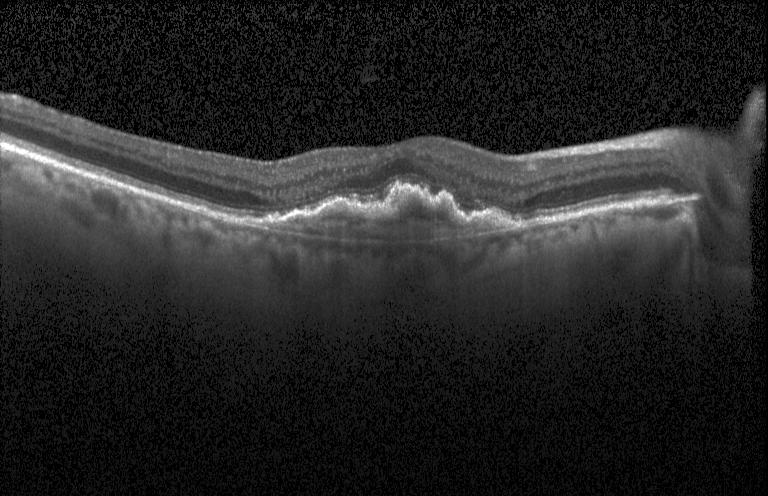

Diagnosis: choroidal neovascularization (CNV).